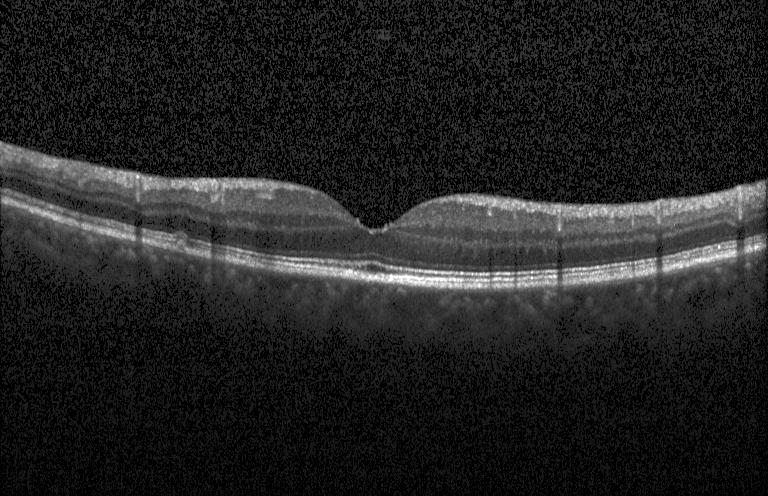 Macular OCT: no choroidal neovascularization, no diabetic macular edema, and no drusen.